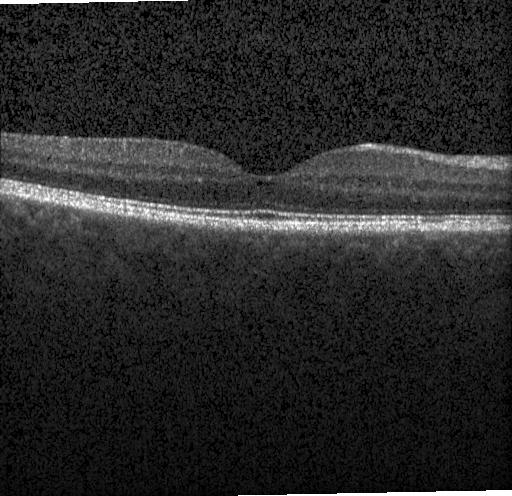

This B-scan demonstrates no choroidal neovascularization, no diabetic macular edema, and no drusen.